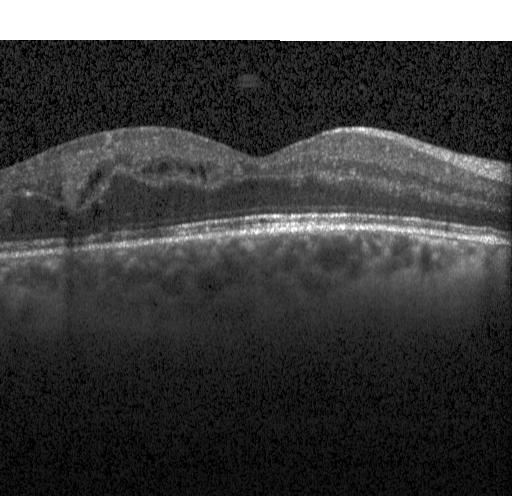
Optical coherence tomography scan.
Assessment: diabetic macular edema (DME).